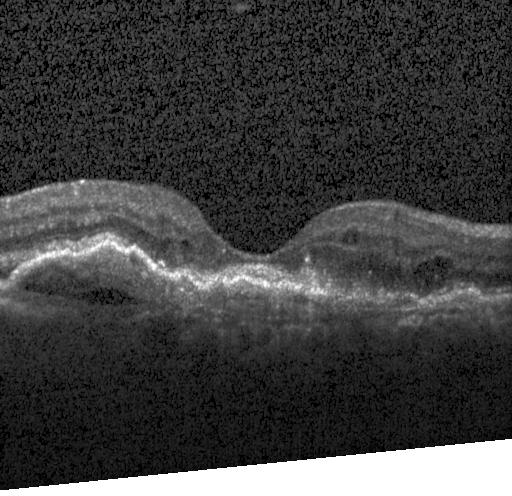 Macular OCT demonstrating a choroidal neovascular membrane.